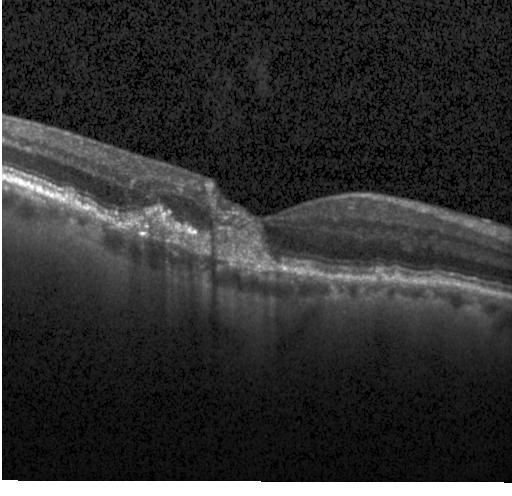

Optical coherence tomography B-scan. Finding: choroidal neovascularization (CNV).